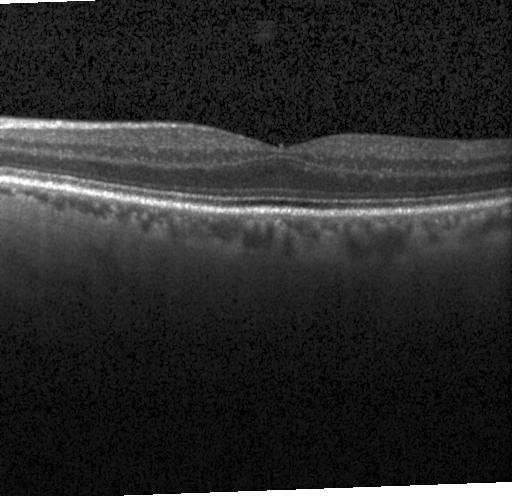
Optical coherence tomography B-scan — Finding: no choroidal neovascularization, diabetic macular edema, or drusen.